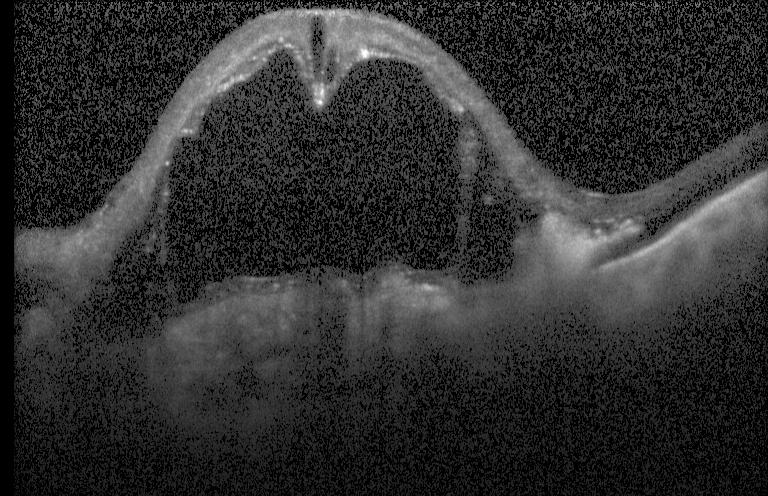

Macular OCT: DME.